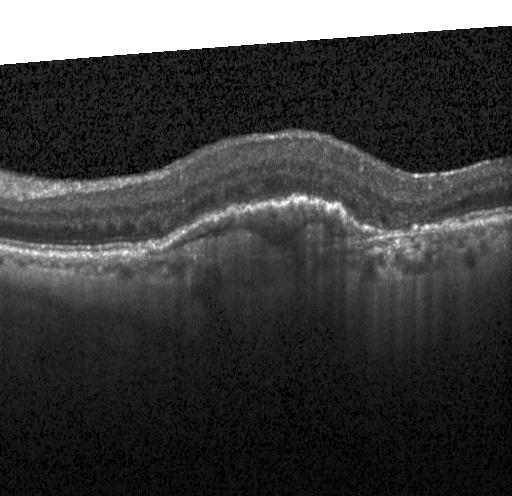

OCT B-scan; SD-OCT; acquired on a Heidelberg Spectralis. Impression: a choroidal neovascular membrane.